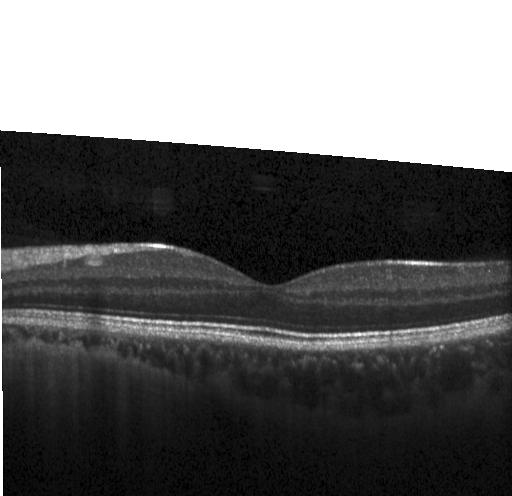
OCT B-scan.
Impression: no choroidal neovascularization, no diabetic macular edema, and no drusen.